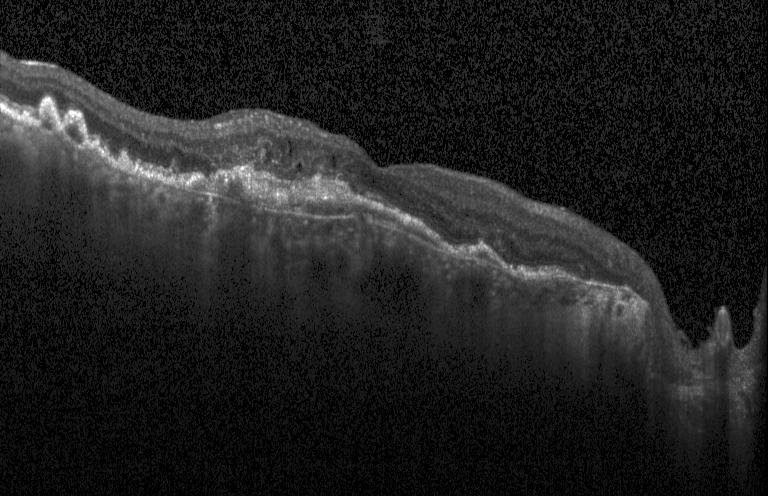 OCT scan showing a choroidal neovascular membrane.